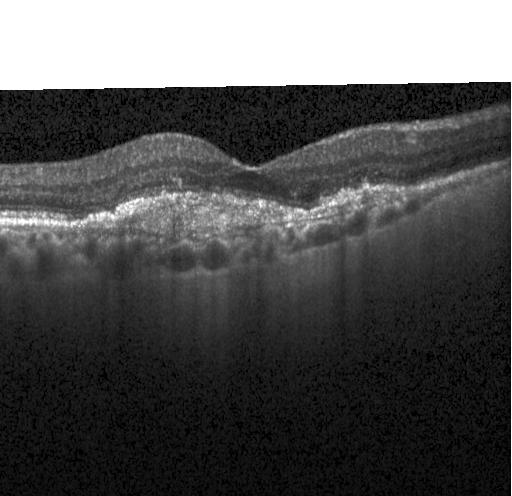

This B-scan demonstrates a choroidal neovascular membrane.